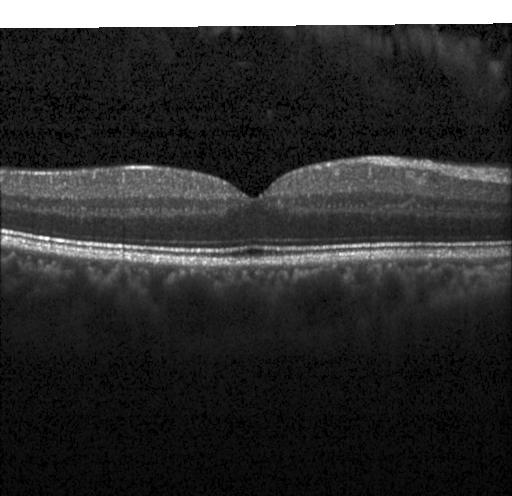
Centered on the fovea · retinal OCT B-scan · acquired on a Heidelberg Spectralis
Impression: no choroidal neovascularization, diabetic macular edema, or drusen.